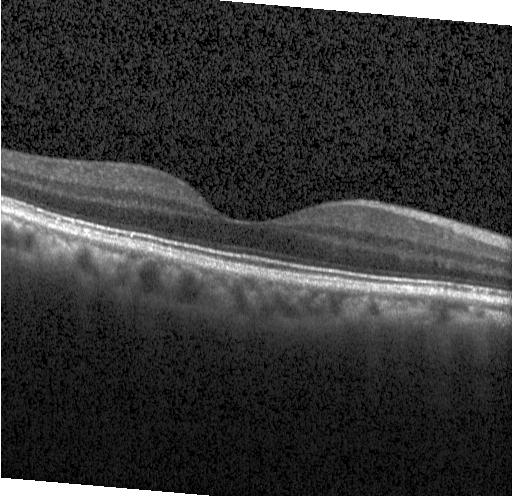

Spectral-domain optical coherence tomography · OCT line scan.
Diagnosis: no choroidal neovascularization, diabetic macular edema, or drusen.